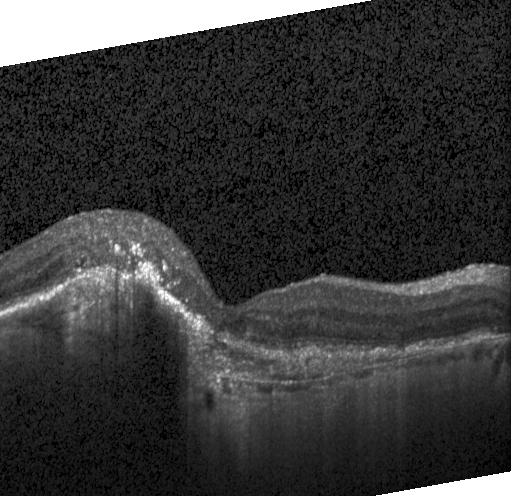
Finding: choroidal neovascularization (CNV).